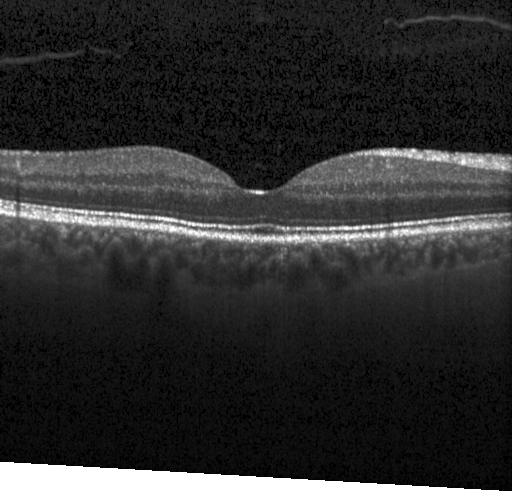
Finding: no choroidal neovascularization, no diabetic macular edema, and no drusen.